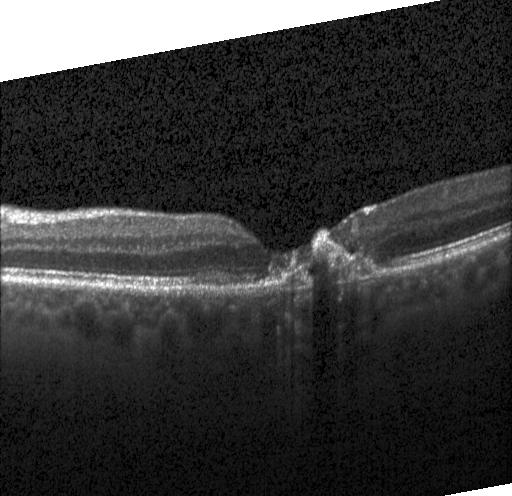
OCT B-scan. Through the macula. Acquired on a Heidelberg Spectralis.
Impression: choroidal neovascularization (CNV).